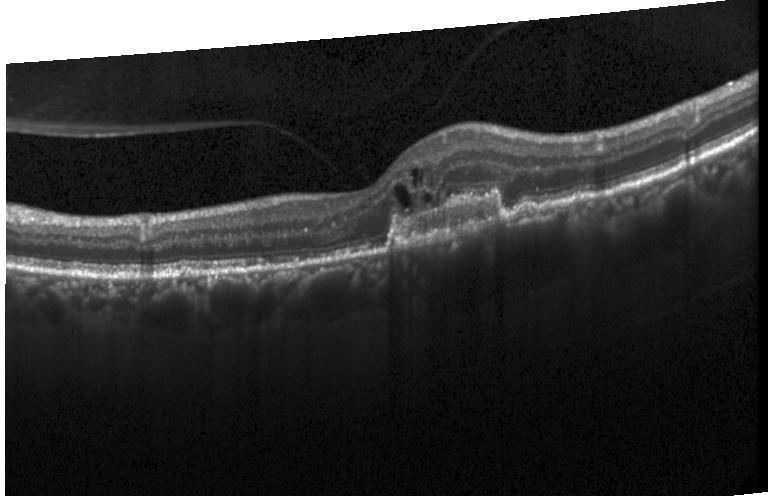

Retinal OCT cross-section — Dx: a choroidal neovascular membrane.